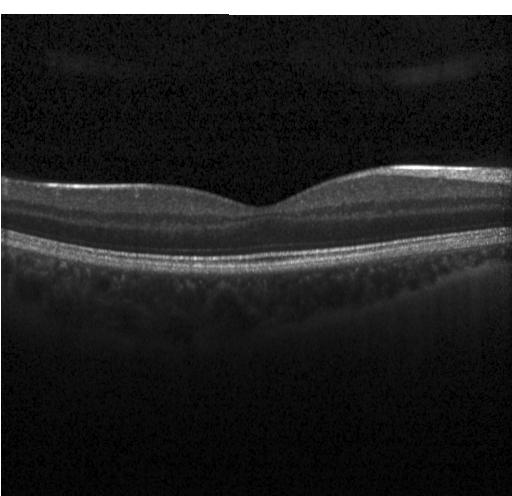
Acquired on a Heidelberg Spectralis. Centered on the fovea. Spectral-domain OCT. Optical coherence tomography scan.
Finding: neither CNV, DME, nor drusen.